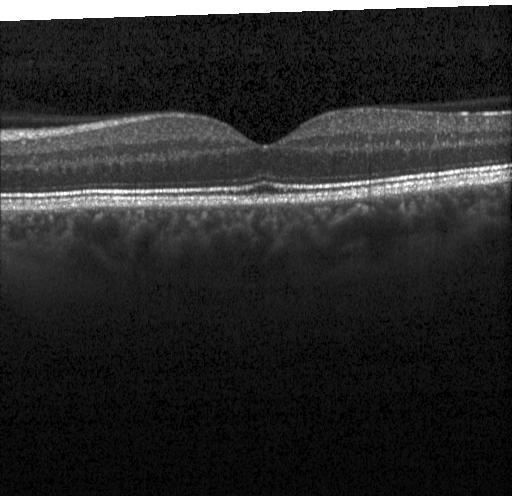 Fovea-centered, retinal OCT B-scan — Macular OCT: neither choroidal neovascularization, diabetic macular edema, nor drusen.